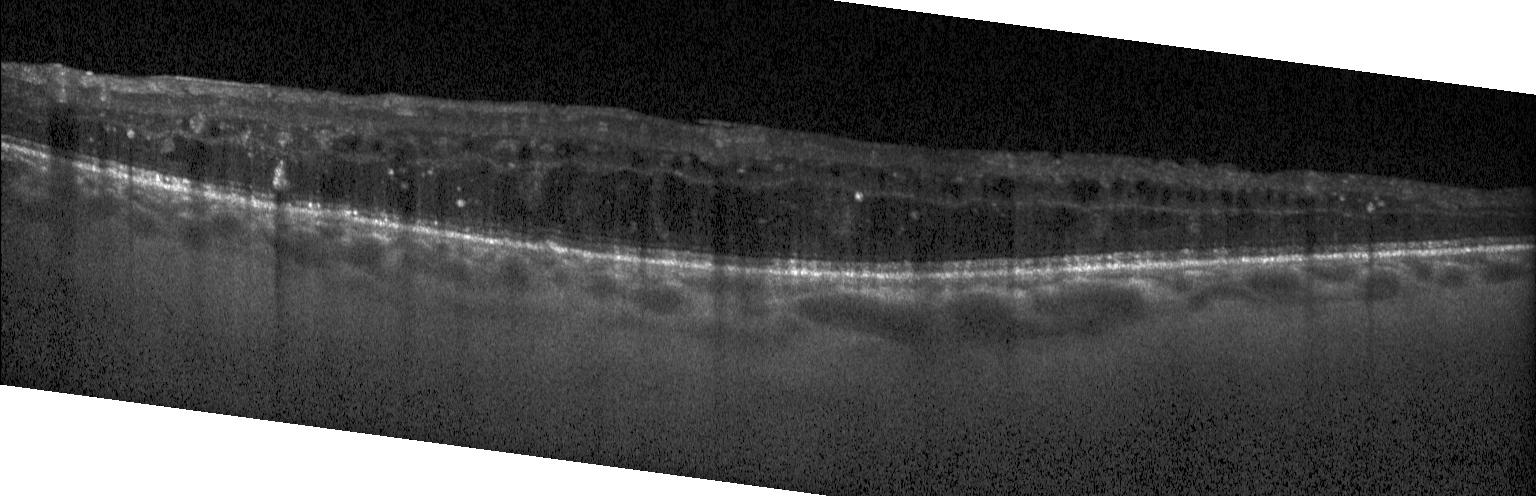 OCT line scan. Heidelberg Spectralis. Impression: DME.